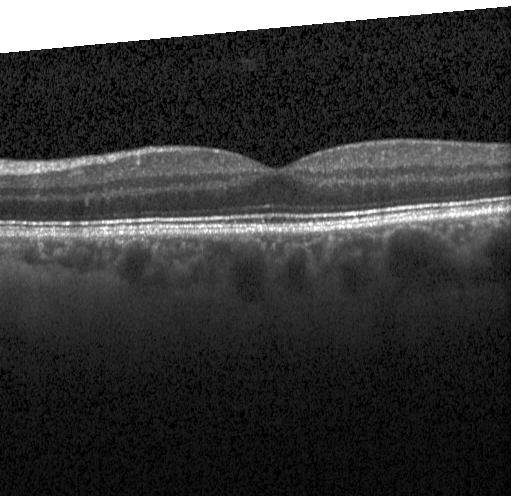 Finding: no evidence of choroidal neovascularization, diabetic macular edema, or drusen.